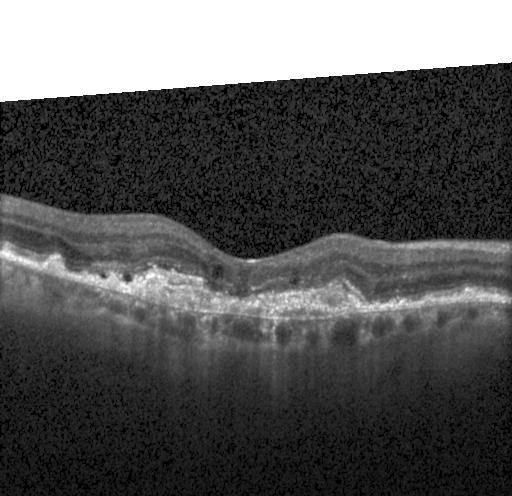 Diagnosis: choroidal neovascularization (CNV).